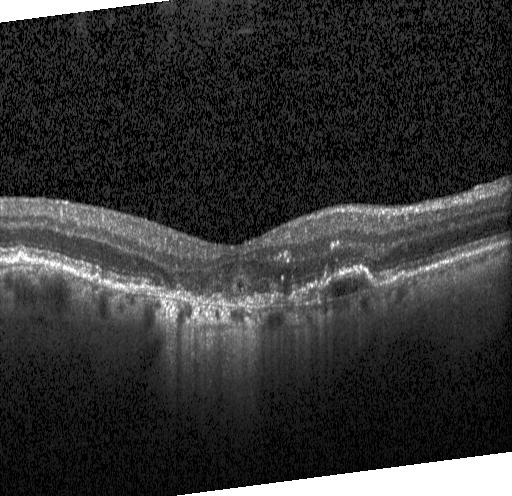
OCT B-scan, instrument: Heidelberg Spectralis
A choroidal neovascular membrane.